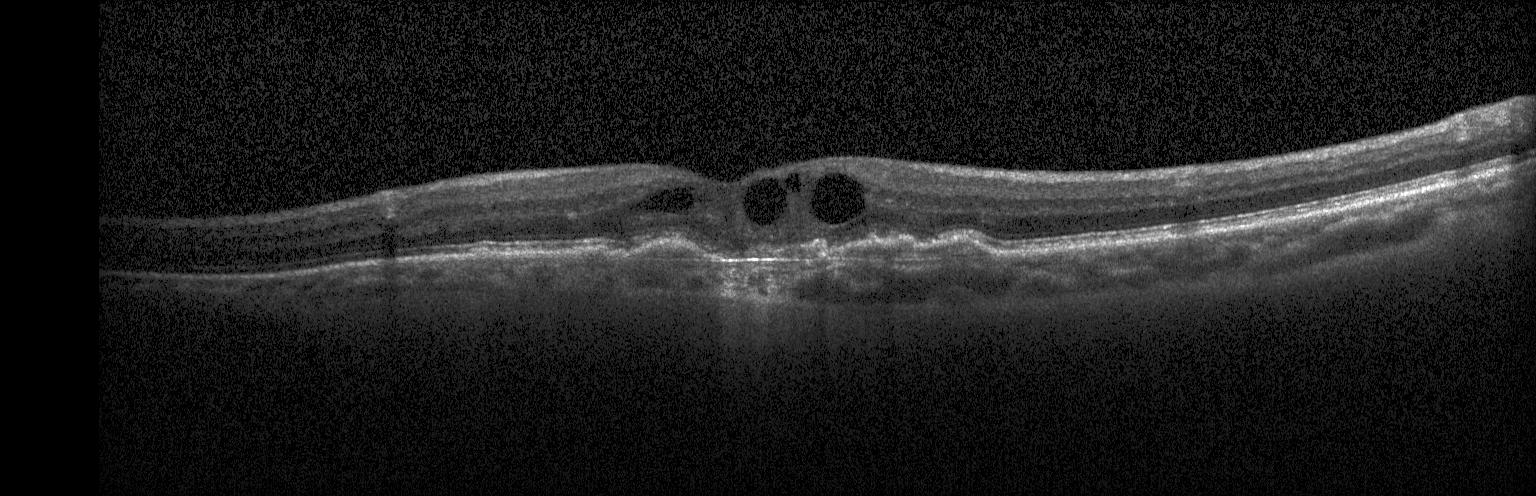 Retinal OCT cross-section; SD-OCT; Heidelberg Spectralis. Impression: a choroidal neovascular membrane.